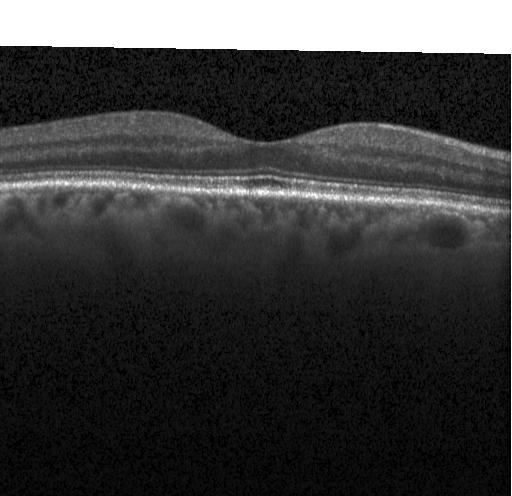

OCT B-scan. Finding: neither choroidal neovascularization, diabetic macular edema, nor drusen.